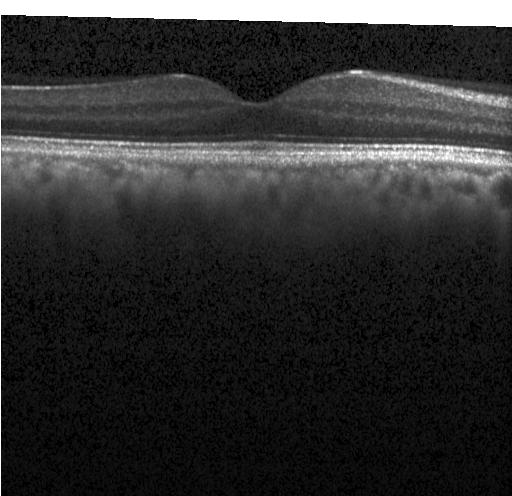

Optical coherence tomography scan — OCT finding: no evidence of CNV, DME, or drusen.